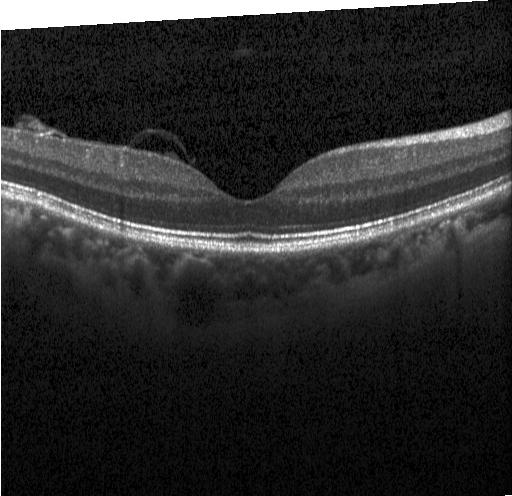 Retinal OCT cross-section showing no choroidal neovascularization, no diabetic macular edema, and no drusen.